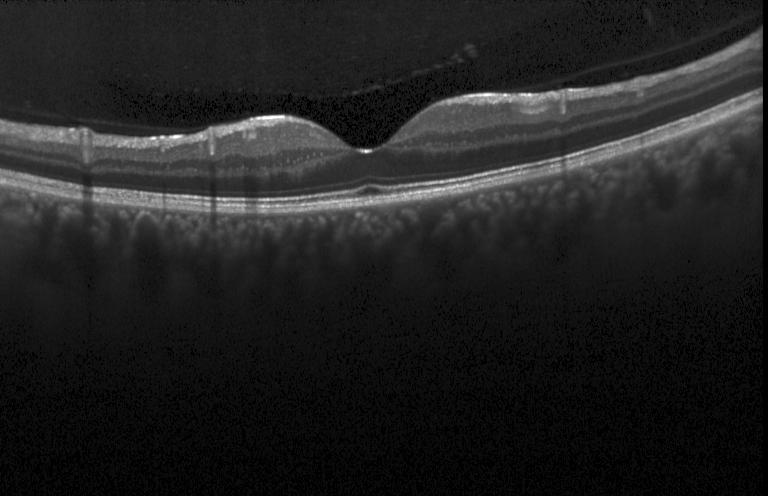

SD-OCT; Heidelberg Spectralis OCT system; retinal OCT B-scan; through the macula. Diagnosis: no evidence of choroidal neovascularization, diabetic macular edema, or drusen.